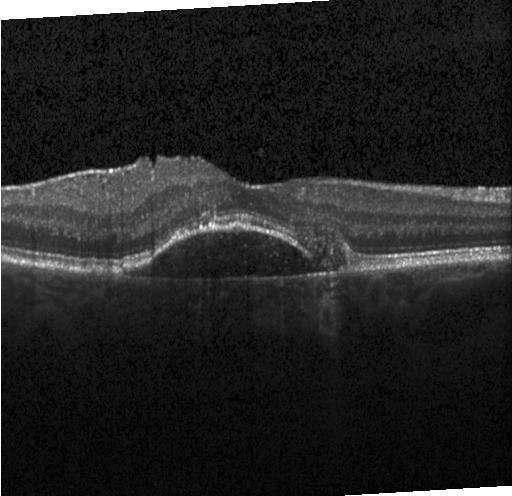 OCT scan showing choroidal neovascularization (CNV).